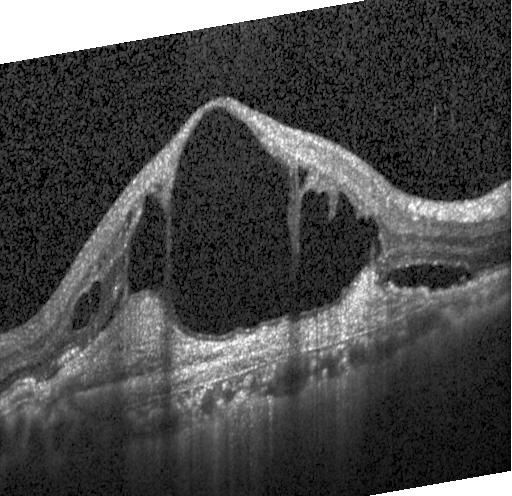 Choroidal neovascularization (CNV).